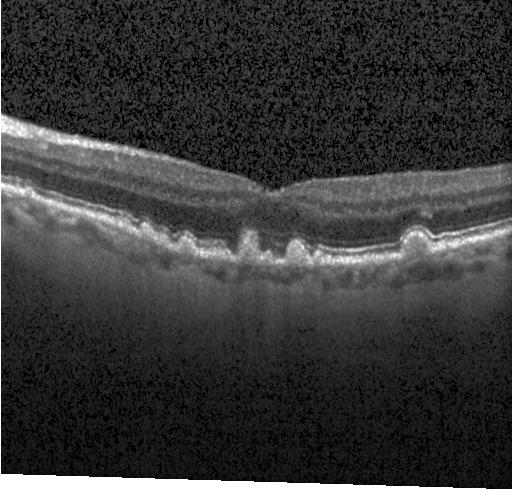

Macular scan. SD-OCT. Retinal OCT B-scan. Dx: multiple drusen.